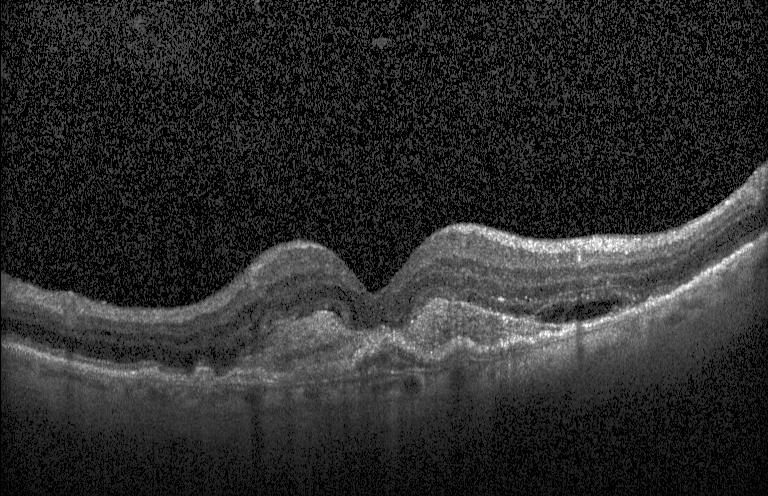

Retinal OCT cross-section.
Choroidal neovascularization (CNV).